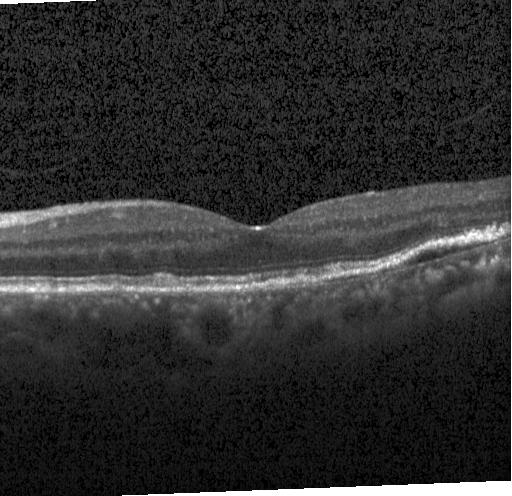 OCT finding: choroidal neovascularization.